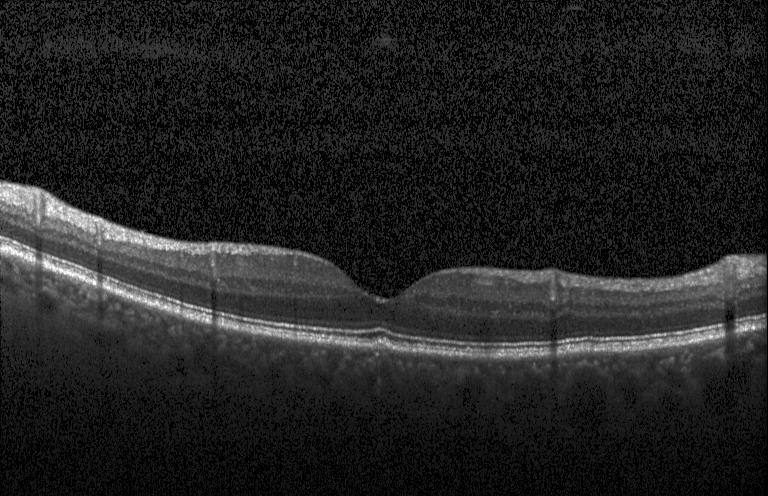 Horizontal scan through the fovea · retinal OCT B-scan — OCT finding: no evidence of choroidal neovascularization, diabetic macular edema, or drusen.